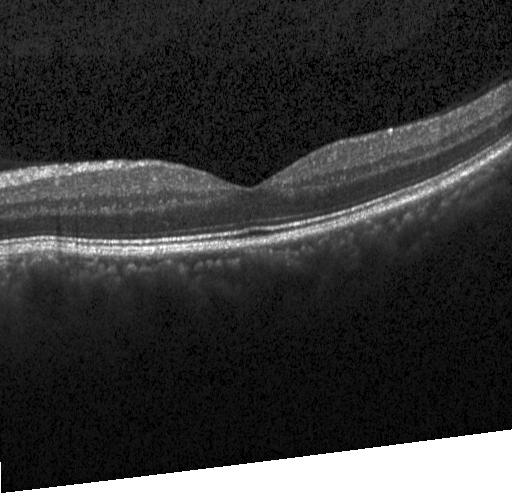

OCT line scan. Assessment: no choroidal neovascularization, diabetic macular edema, or drusen.